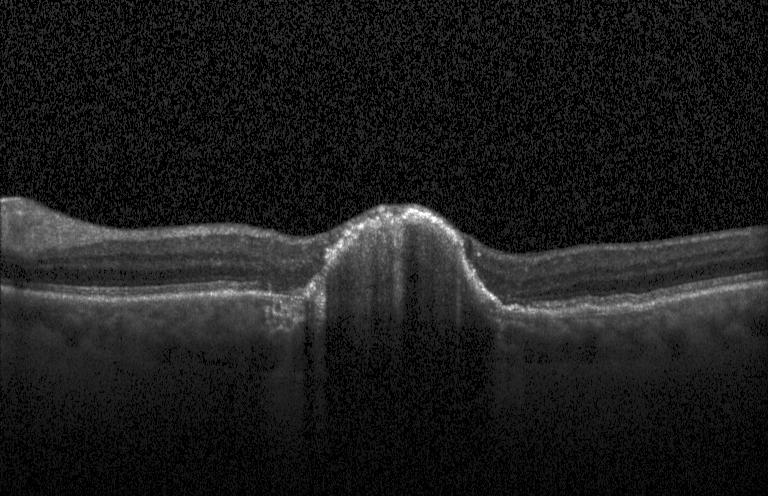 Spectral-domain optical coherence tomography. Heidelberg Spectralis OCT system. Retinal OCT cross-section
Impression: choroidal neovascularization.